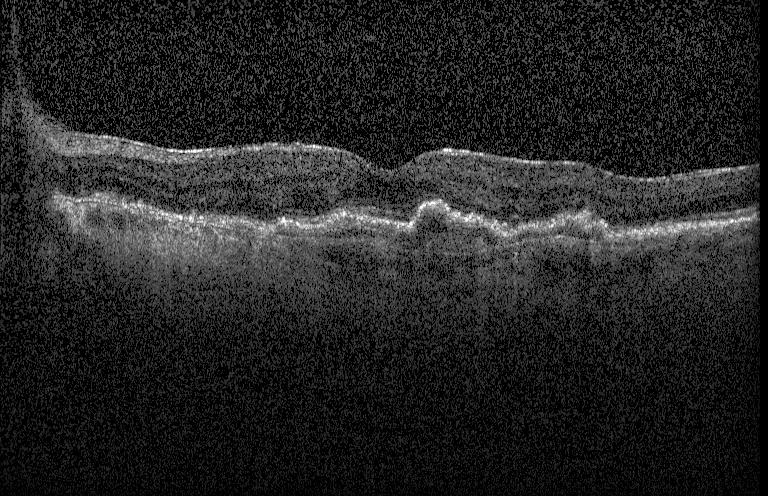

Diagnosis: choroidal neovascularization (CNV).